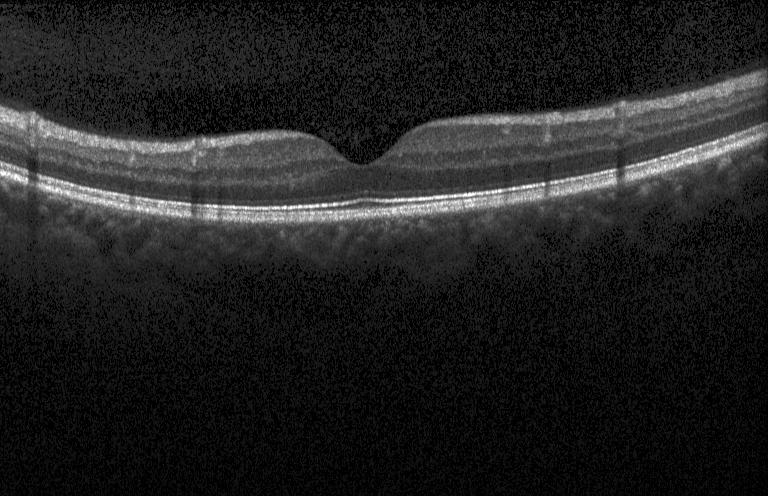
Fovea-centered; retinal OCT cross-section
This B-scan demonstrates no CNV, DME, or drusen.